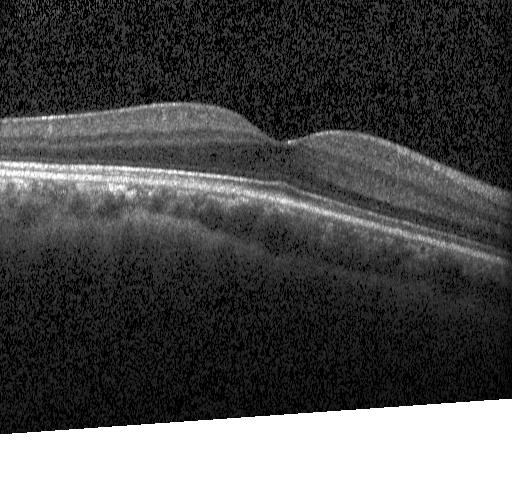
Instrument: Heidelberg Spectralis; OCT line scan. Dx: neither choroidal neovascularization, diabetic macular edema, nor drusen.